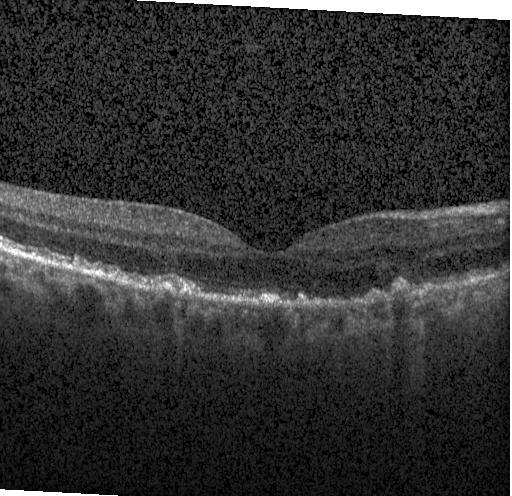

Retinal OCT B-scan — Diagnosis: multiple drusen.